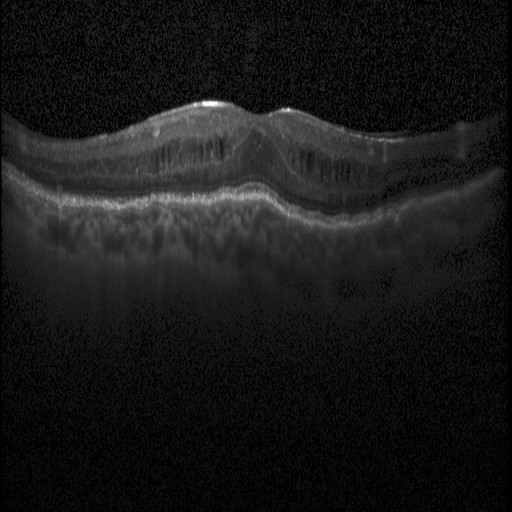

Optical coherence tomography scan, acquired on a Heidelberg Spectralis — Diagnosis: DME.